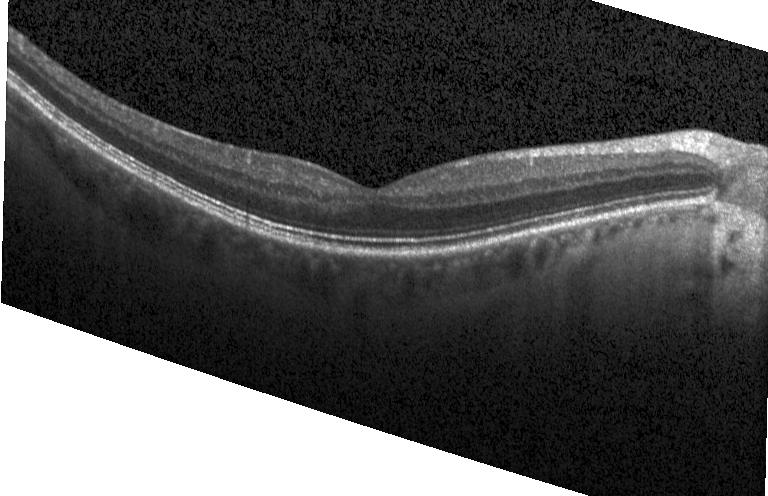 OCT finding: neither choroidal neovascularization, diabetic macular edema, nor drusen.